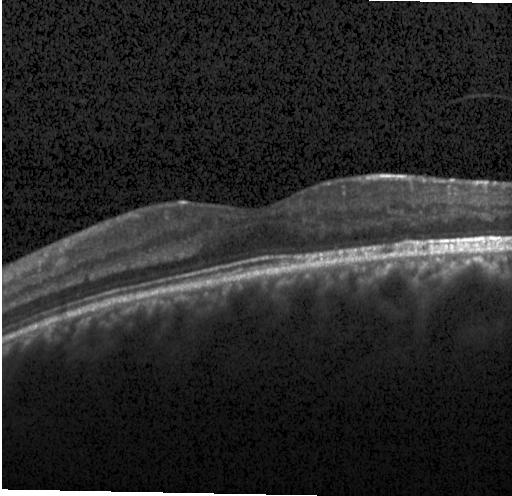

No evidence of choroidal neovascularization, diabetic macular edema, or drusen.